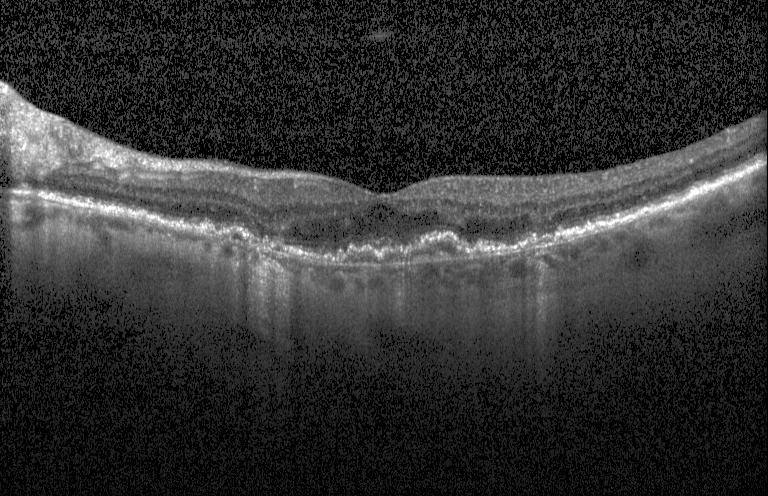 Optical coherence tomography B-scan, SD-OCT, Heidelberg Spectralis — Impression: CNV.